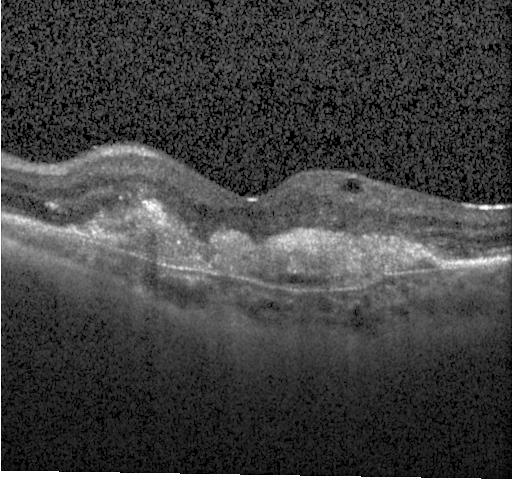
Heidelberg Spectralis OCT system. OCT B-scan. Assessment: a choroidal neovascular membrane.